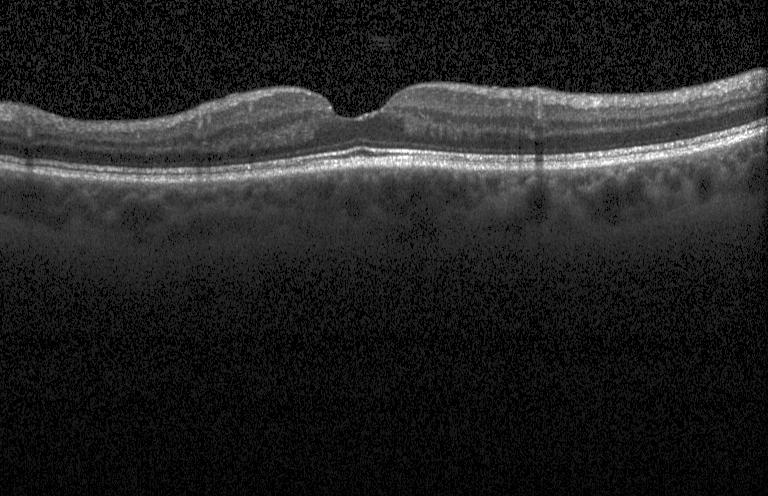
Macular OCT: no choroidal neovascularization, diabetic macular edema, or drusen.